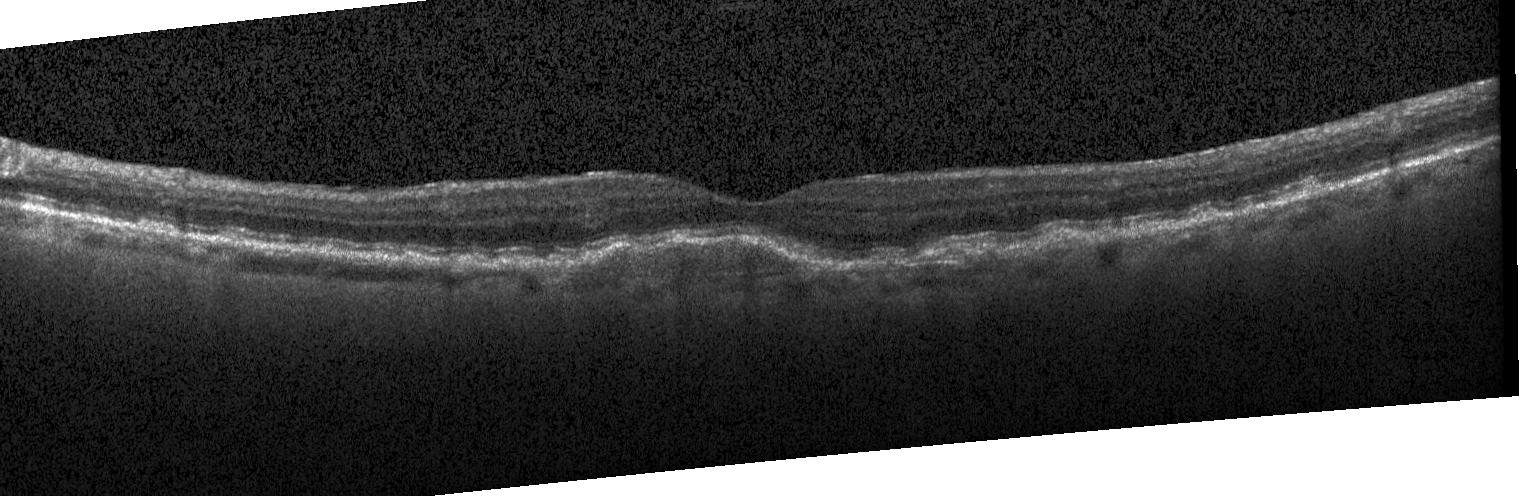
OCT B-scan.
Assessment: a choroidal neovascular membrane.